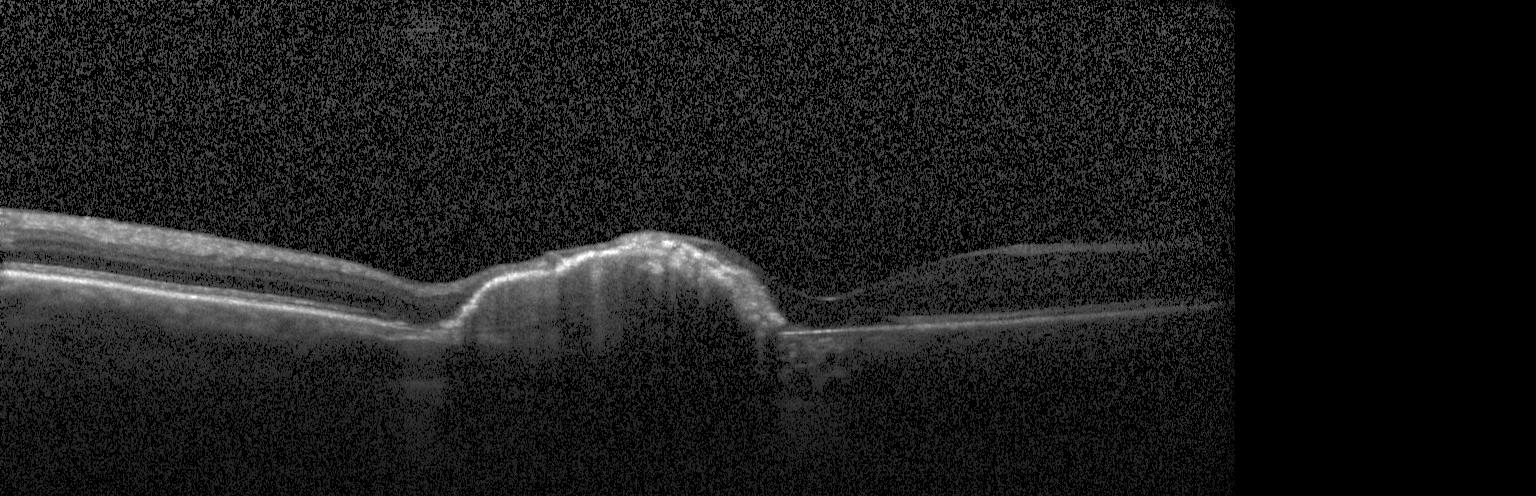
OCT B-scan, Heidelberg Spectralis OCT system, centered on the fovea, spectral-domain OCT
This B-scan demonstrates choroidal neovascularization.